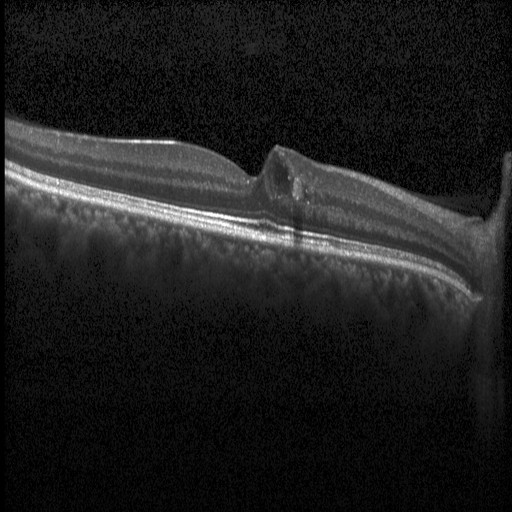

Optical coherence tomography scan — Impression: DME.